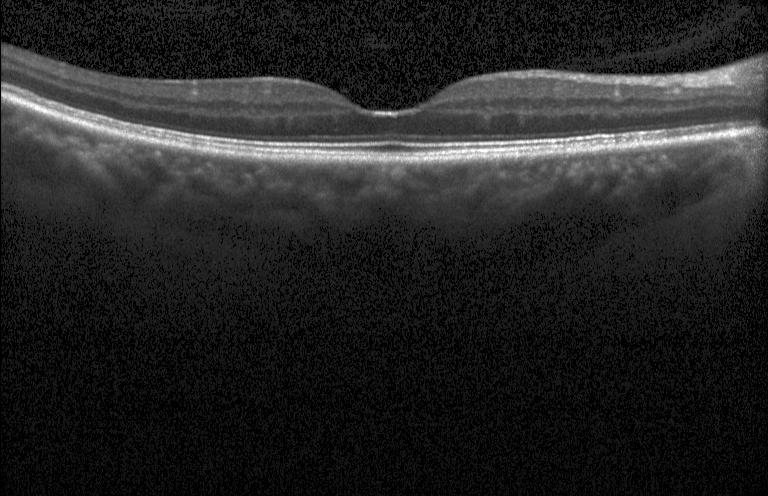
Optical coherence tomography B-scan · macular scan. Impression: no evidence of choroidal neovascularization, diabetic macular edema, or drusen.